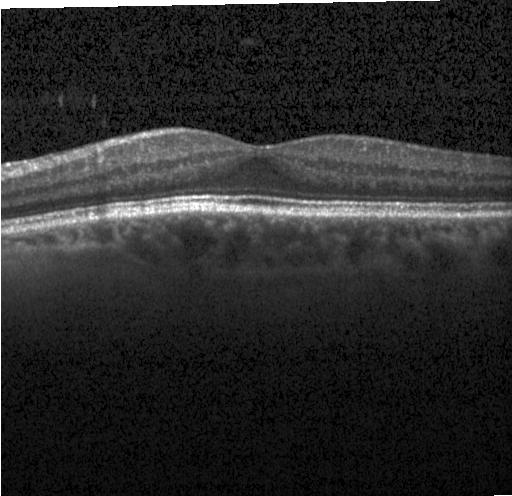
Impression: no evidence of choroidal neovascularization, diabetic macular edema, or drusen.